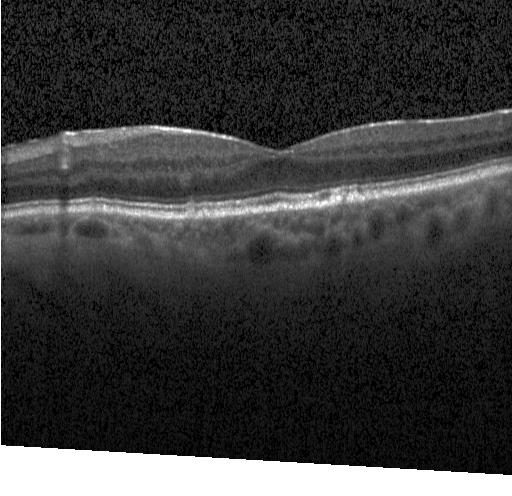 Acquired on a Heidelberg Spectralis; spectral-domain OCT; retinal OCT cross-section.
Sub-RPE drusenoid deposits.